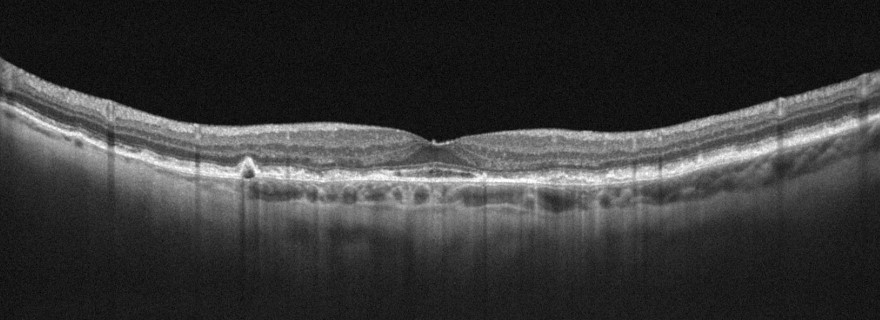
Optical coherence tomography B-scan · Optovue Avanti RTVue XR · fovea-centered. Age-related macular degeneration (AMD).